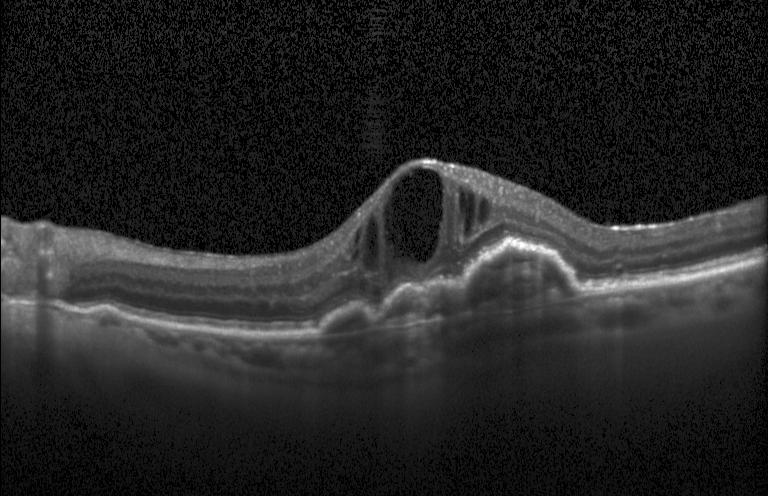

A choroidal neovascular membrane.